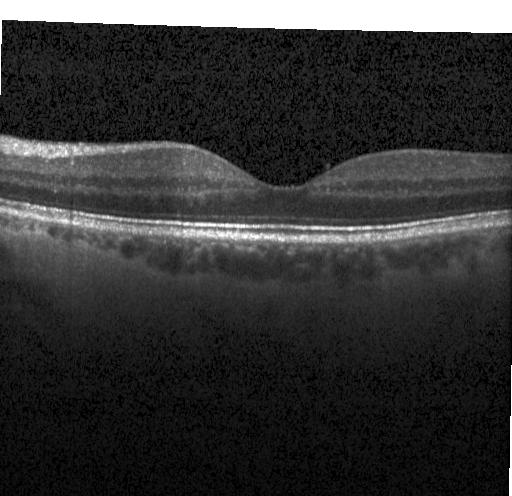

Finding: no choroidal neovascularization, diabetic macular edema, or drusen.